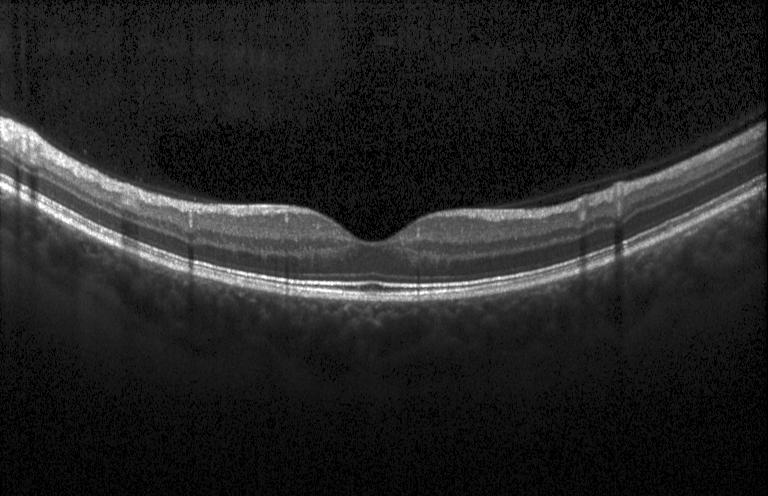

OCT B-scan · Heidelberg Spectralis — Impression: no evidence of choroidal neovascularization, diabetic macular edema, or drusen.